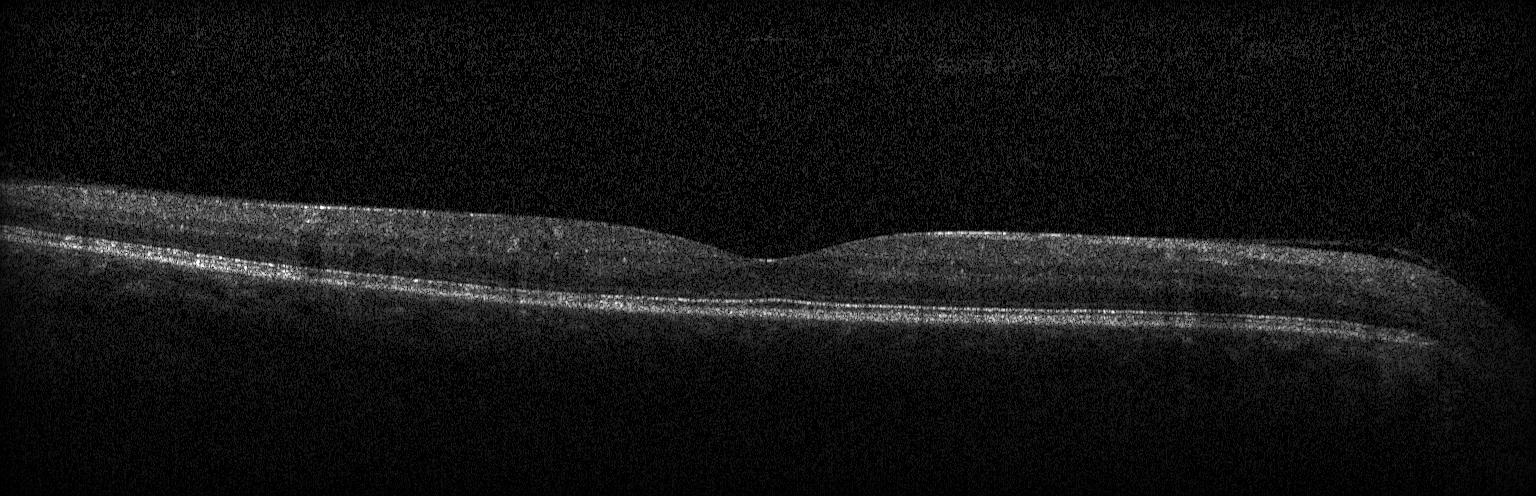

OCT scan showing no evidence of choroidal neovascularization, diabetic macular edema, or drusen.